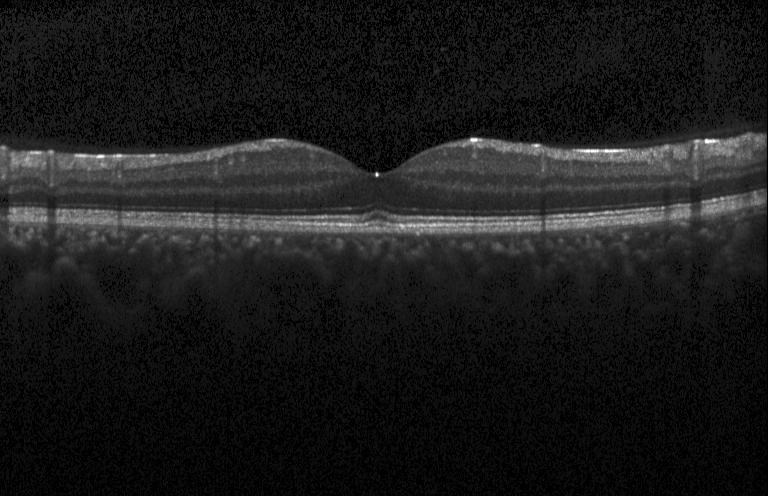

Macular scan. Retinal OCT B-scan. Instrument: Heidelberg Spectralis. Spectral-domain OCT. No choroidal neovascularization, diabetic macular edema, or drusen.